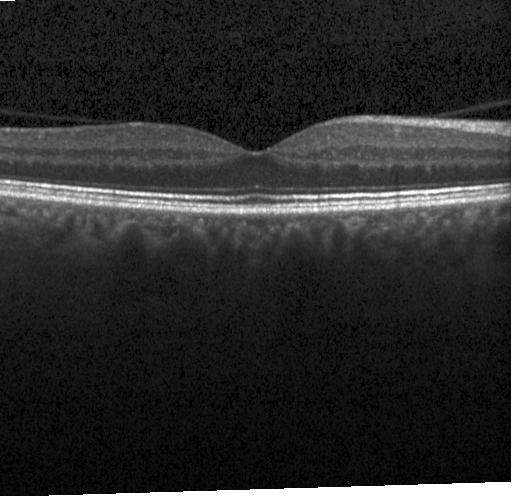 No choroidal neovascularization, diabetic macular edema, or drusen.